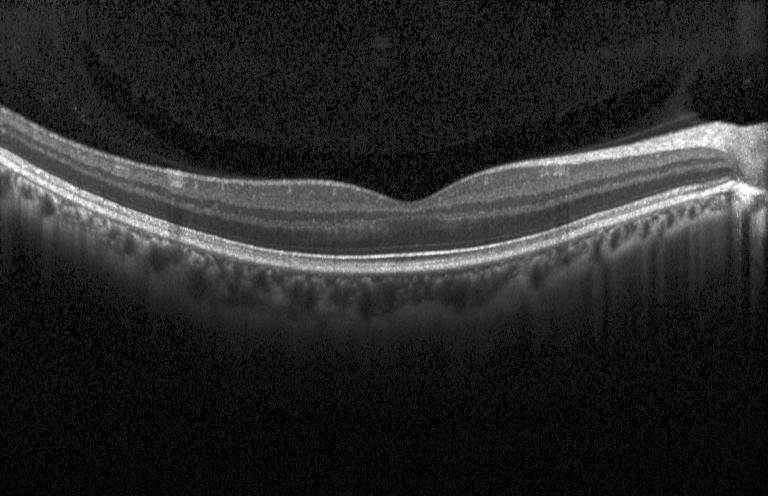
Retinal OCT B-scan — The scan shows neither choroidal neovascularization, diabetic macular edema, nor drusen.